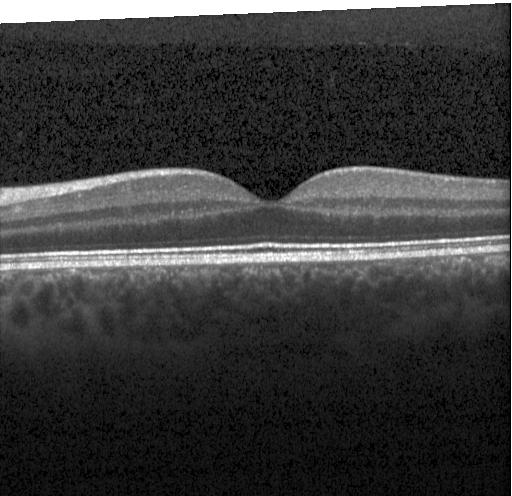
Optical coherence tomography scan. Centered on the fovea — The scan shows neither choroidal neovascularization, diabetic macular edema, nor drusen.